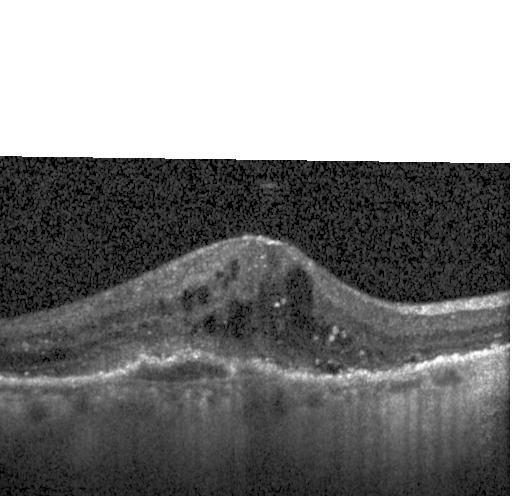
Retinal OCT B-scan · macular scan · instrument: Heidelberg Spectralis
Impression: a choroidal neovascular membrane.